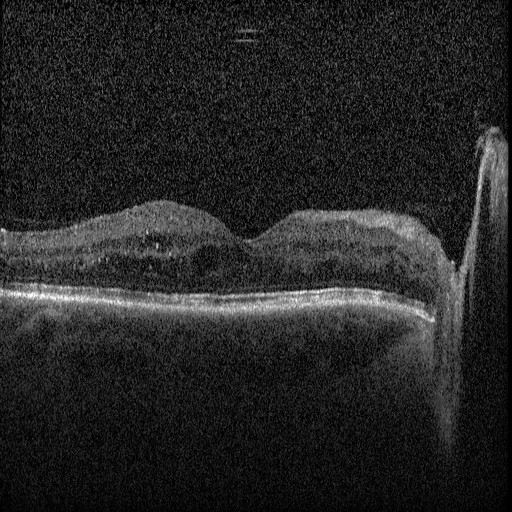
OCT finding: DME.